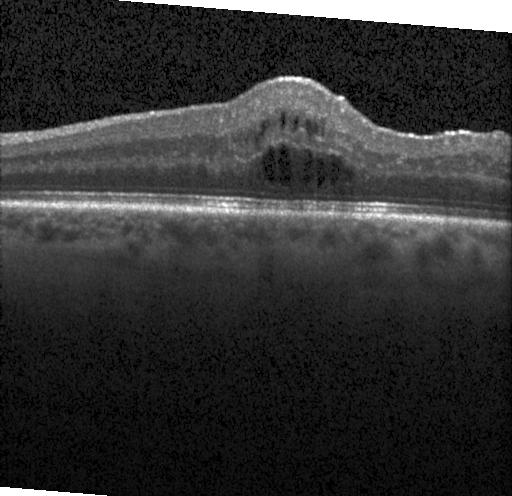
OCT finding: DME.